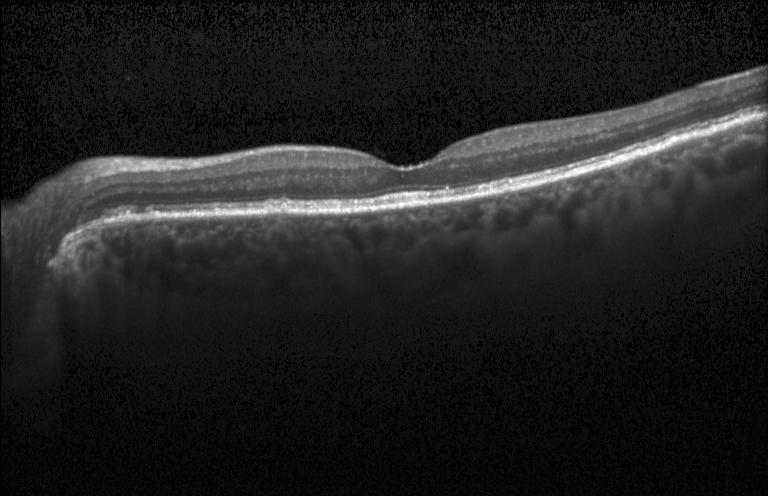

Finding: drusen.